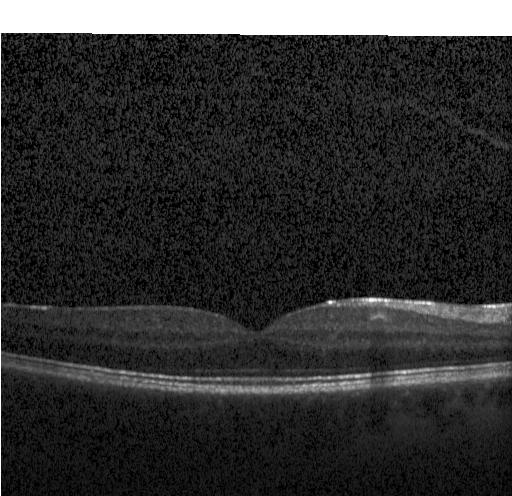
OCT B-scan, centered on the fovea — This B-scan demonstrates no choroidal neovascularization, no diabetic macular edema, and no drusen.